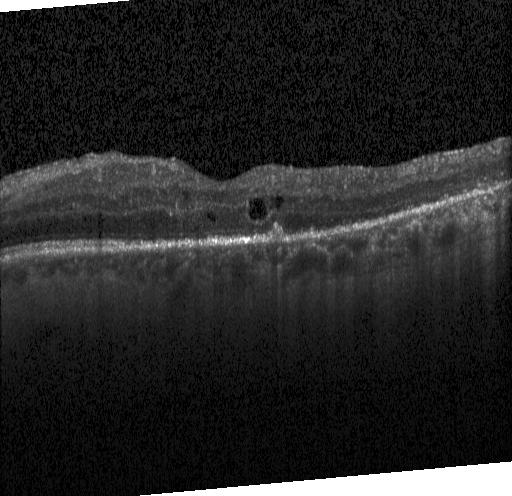
Fovea-centered · SD-OCT · optical coherence tomography B-scan.
Finding: diabetic macular edema (DME).